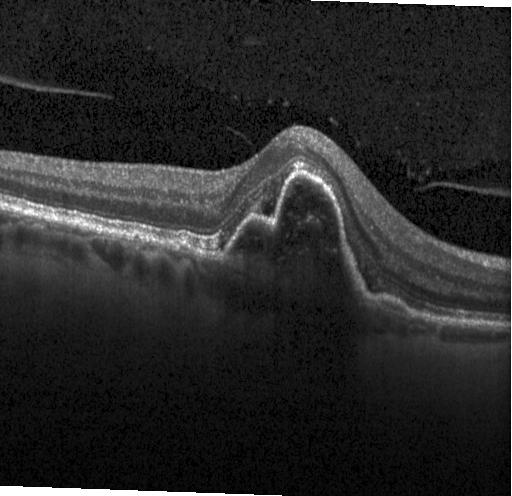

This B-scan demonstrates choroidal neovascularization.